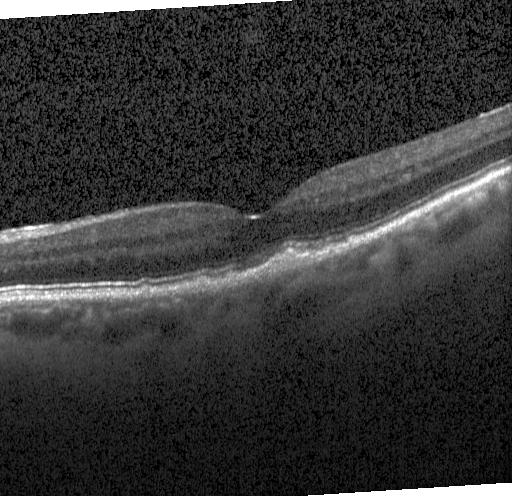
This B-scan demonstrates drusen.